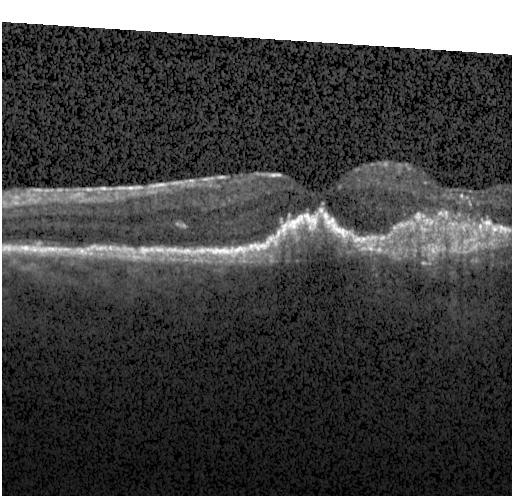
Instrument: Heidelberg Spectralis, fovea-centered, optical coherence tomography B-scan.
The scan shows choroidal neovascularization.